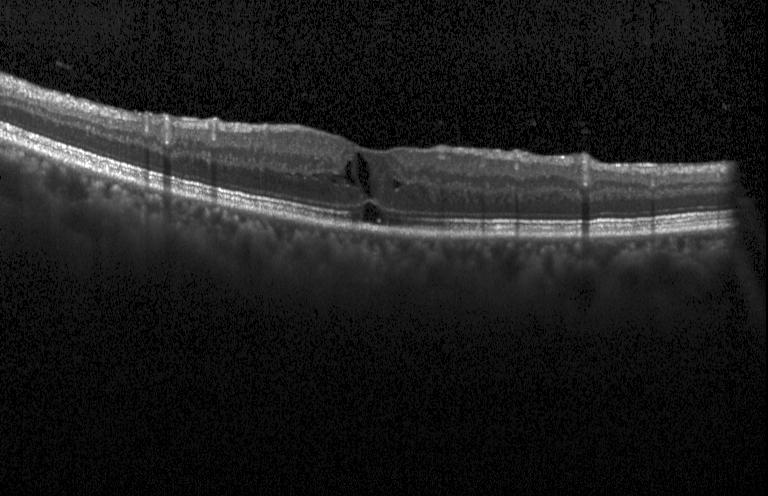
Horizontal scan through the fovea · Heidelberg Spectralis OCT system · optical coherence tomography scan · spectral-domain optical coherence tomography. Impression: DME.